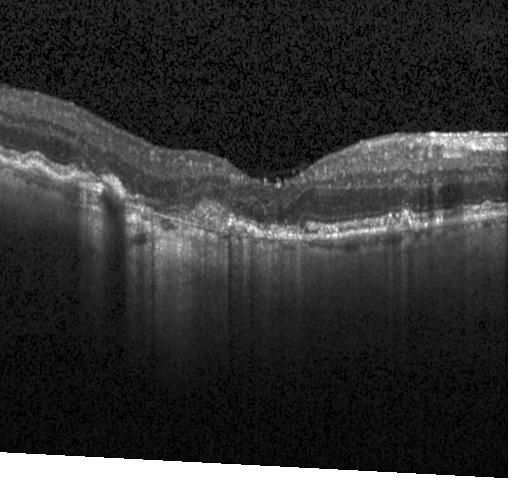
Optical coherence tomography B-scan.
Dx: a choroidal neovascular membrane.